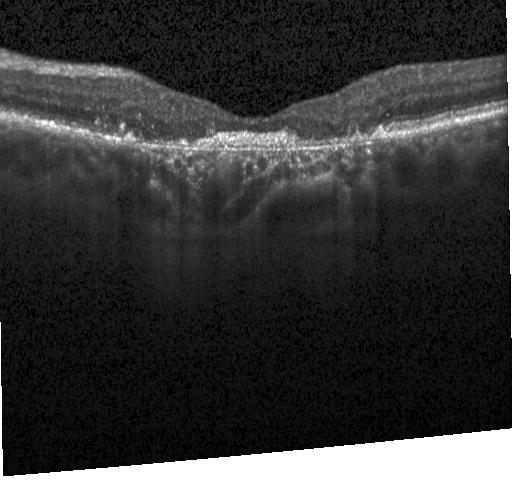 Instrument: Heidelberg Spectralis. Horizontal scan through the fovea. Optical coherence tomography scan. Spectral-domain optical coherence tomography — Impression: a choroidal neovascular membrane.